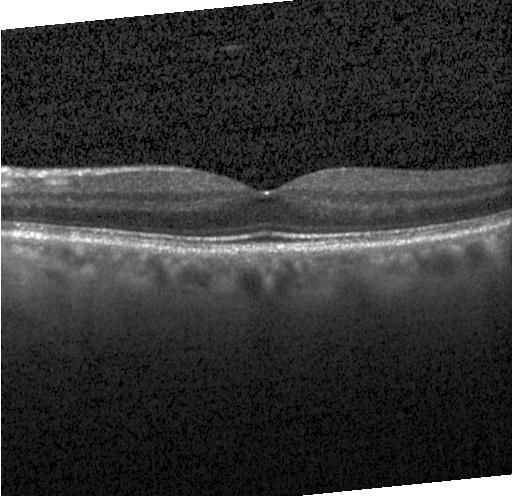
Acquired on a Heidelberg Spectralis, optical coherence tomography scan. OCT finding: no evidence of choroidal neovascularization, diabetic macular edema, or drusen.